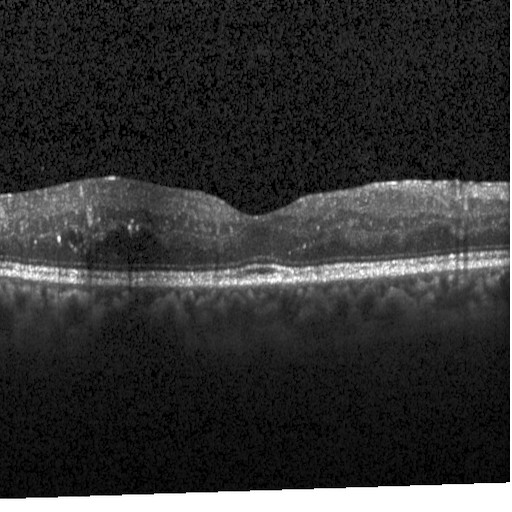
Optical coherence tomography scan, acquired on a Heidelberg Spectralis — Diagnosis: diabetic macular edema (DME).